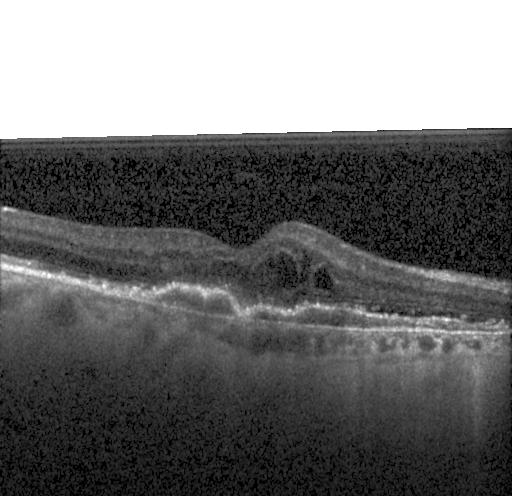

The scan shows choroidal neovascularization.